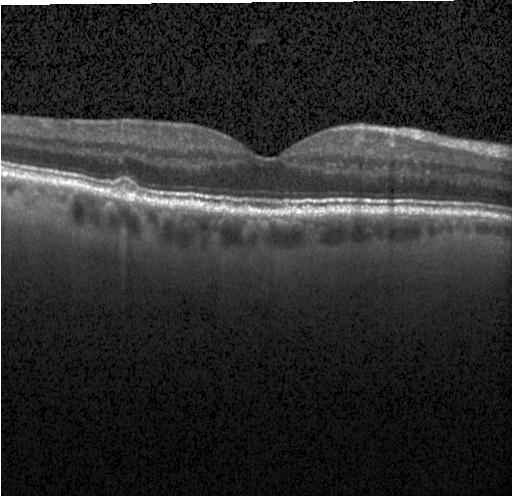 OCT B-scan showing multiple drusen.